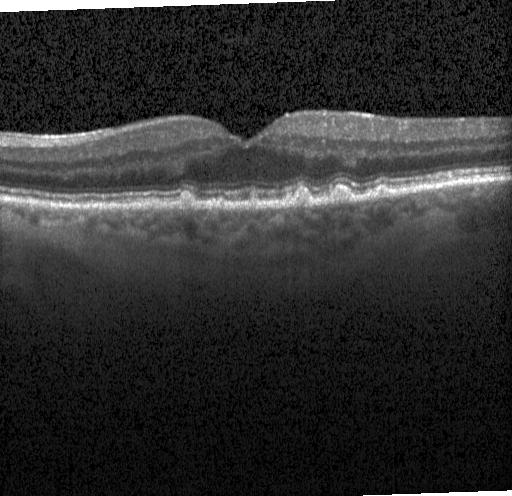
OCT line scan
This B-scan demonstrates sub-RPE drusenoid deposits.